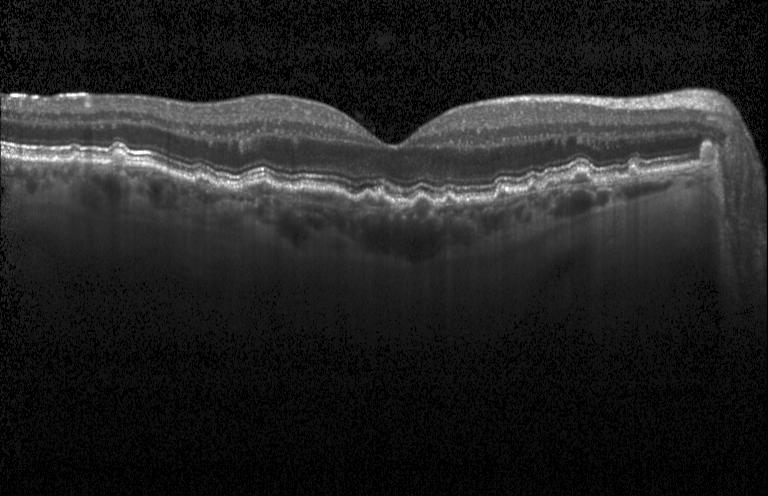 Multiple drusen.